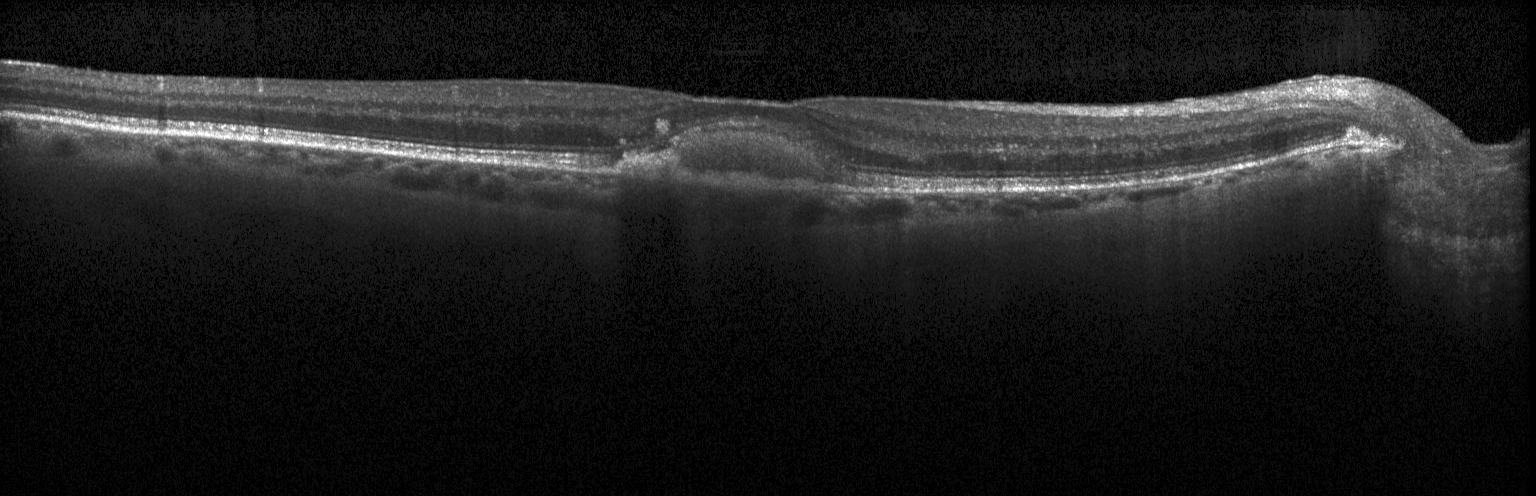

Optical coherence tomography B-scan · through the macula · Heidelberg Spectralis OCT system. Impression: choroidal neovascularization (CNV).